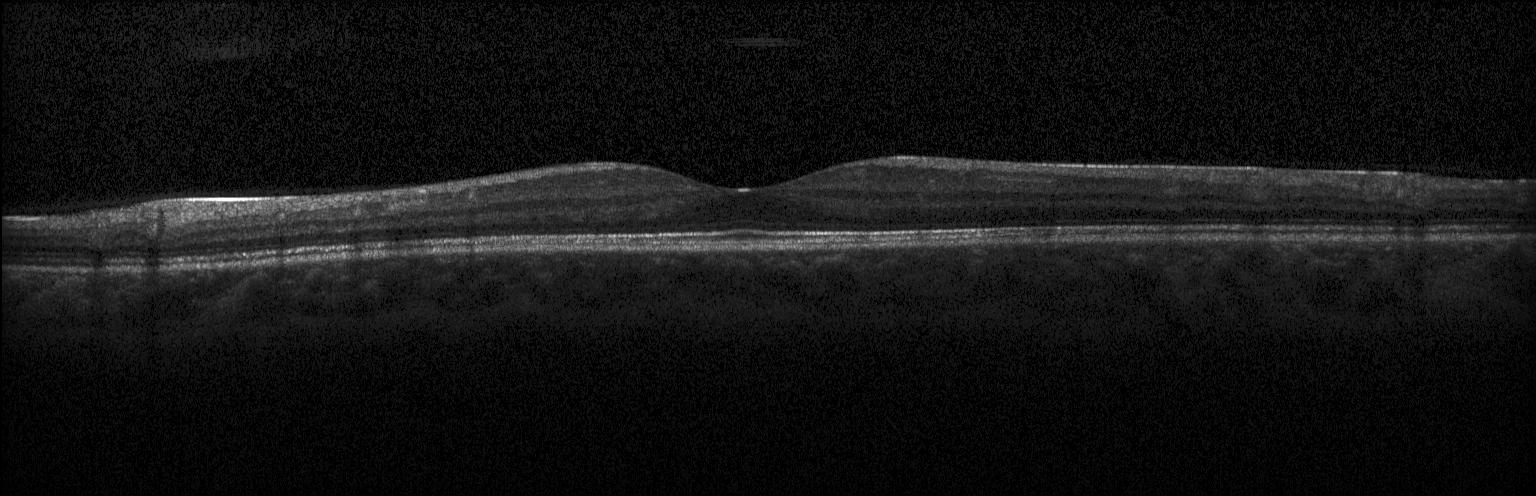
Finding: no CNV, no DME, and no drusen.